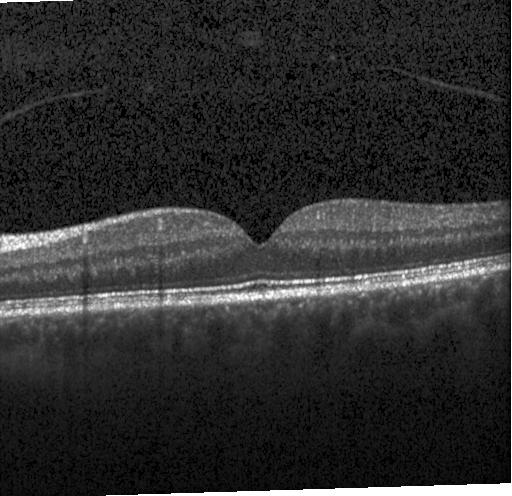
Spectral-domain optical coherence tomography; Heidelberg Spectralis; optical coherence tomography scan; fovea-centered.
Macular OCT: neither choroidal neovascularization, diabetic macular edema, nor drusen.